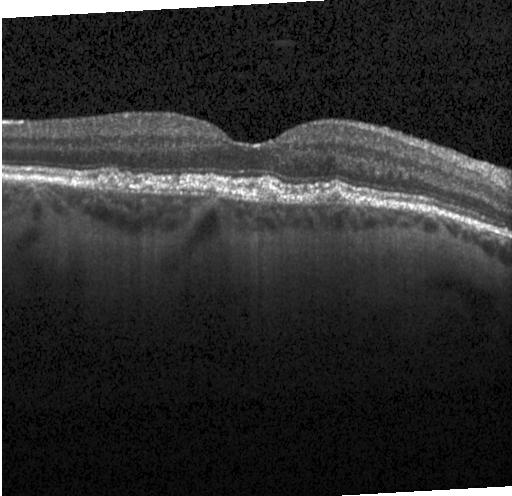

OCT finding: drusen.